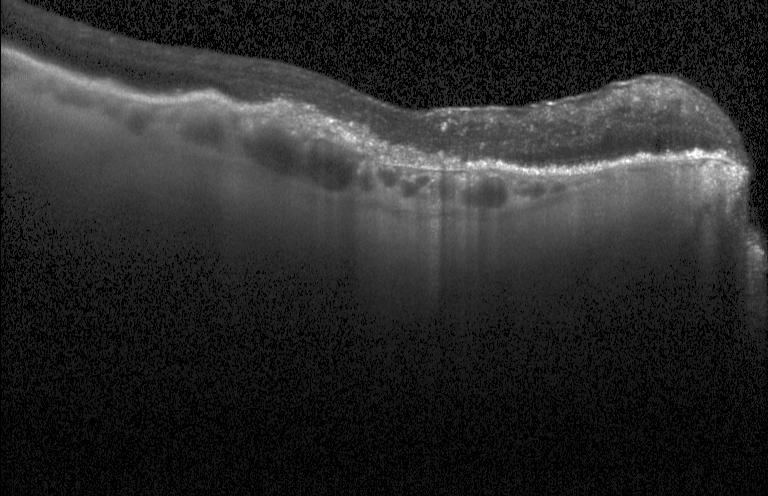 OCT line scan, horizontal scan through the fovea, SD-OCT, Heidelberg Spectralis OCT system.
Finding: a choroidal neovascular membrane.